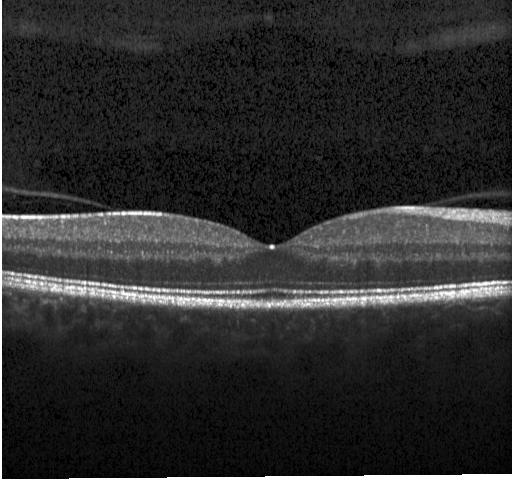 OCT B-scan — Assessment: no evidence of CNV, DME, or drusen.